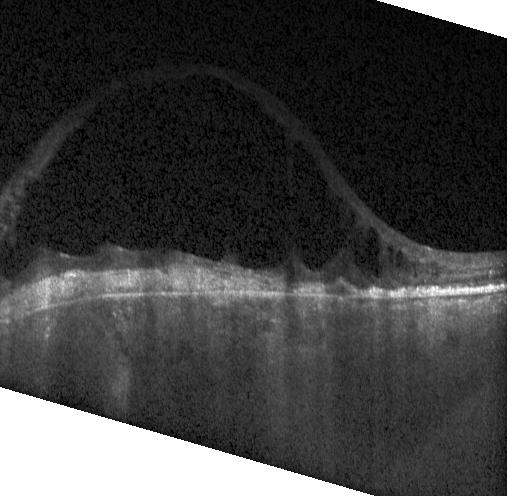
OCT finding: choroidal neovascularization (CNV).